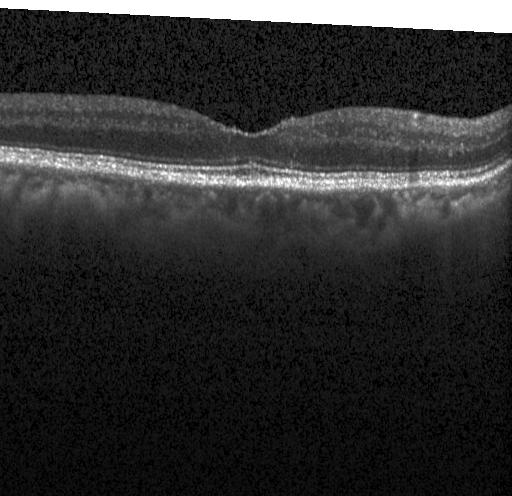 Horizontal scan through the fovea; OCT line scan; spectral-domain optical coherence tomography; acquired on a Heidelberg Spectralis — OCT finding: neither choroidal neovascularization, diabetic macular edema, nor drusen.